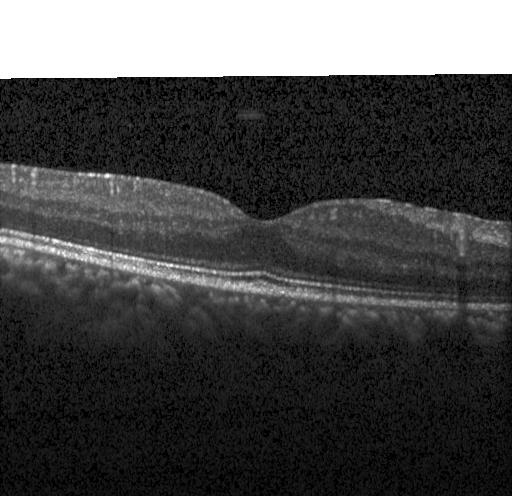
SD-OCT, optical coherence tomography B-scan — Dx: no evidence of choroidal neovascularization, diabetic macular edema, or drusen.